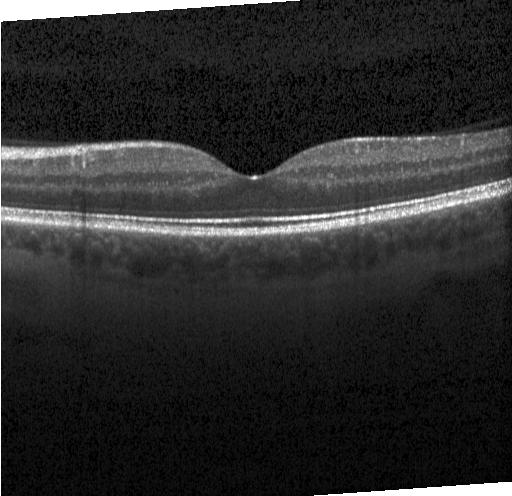 Spectral-domain OCT B-scan: neither choroidal neovascularization, diabetic macular edema, nor drusen.